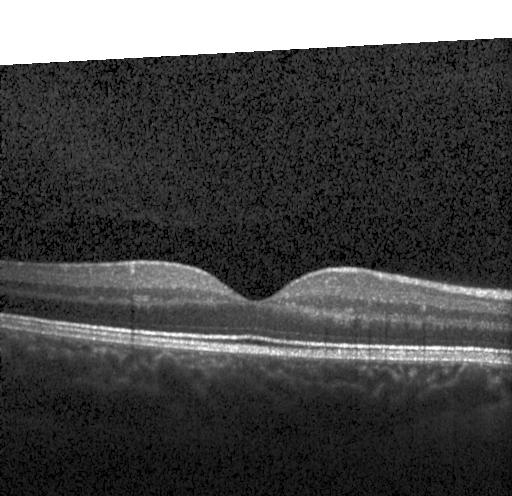 OCT line scan · fovea-centered · acquired on a Heidelberg Spectralis · spectral-domain optical coherence tomography. No choroidal neovascularization, no diabetic macular edema, and no drusen.